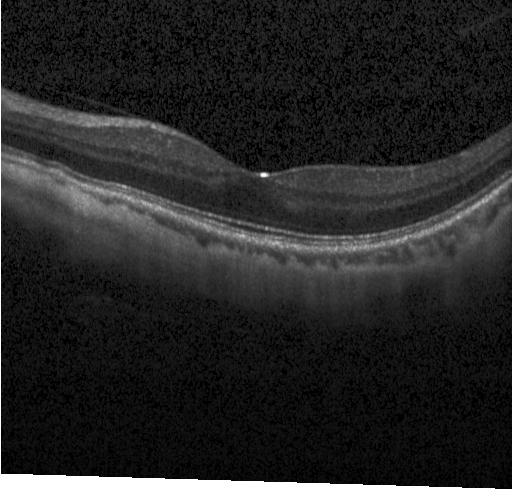 Optical coherence tomography scan, Heidelberg Spectralis
The scan shows neither CNV, DME, nor drusen.